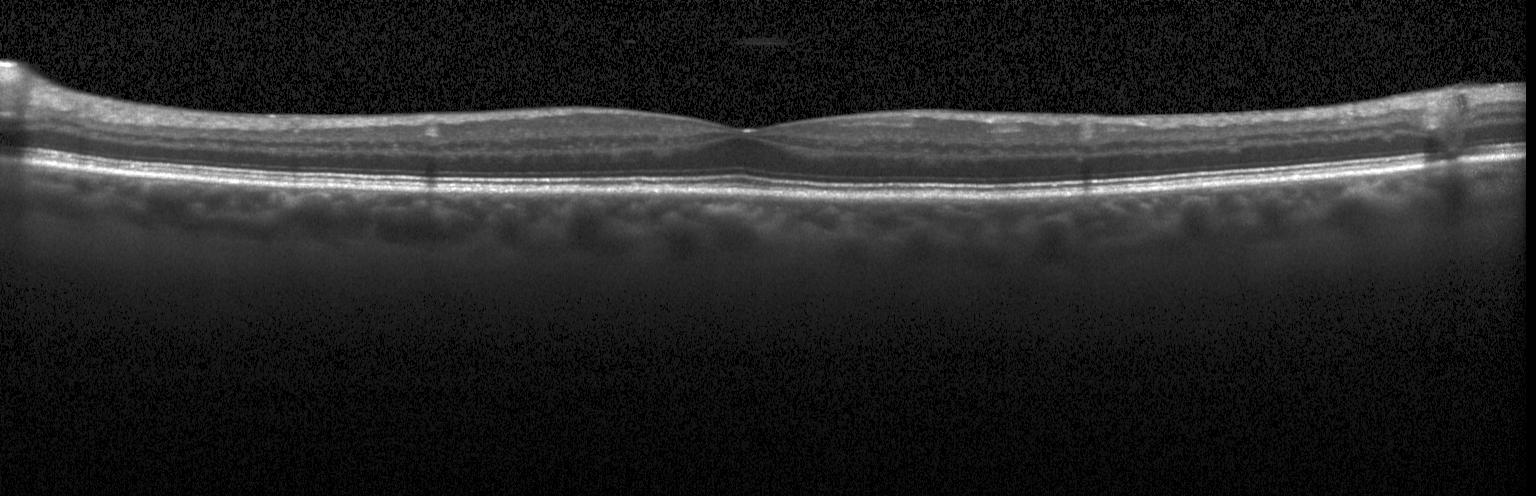

OCT B-scan — Finding: neither choroidal neovascularization, diabetic macular edema, nor drusen.